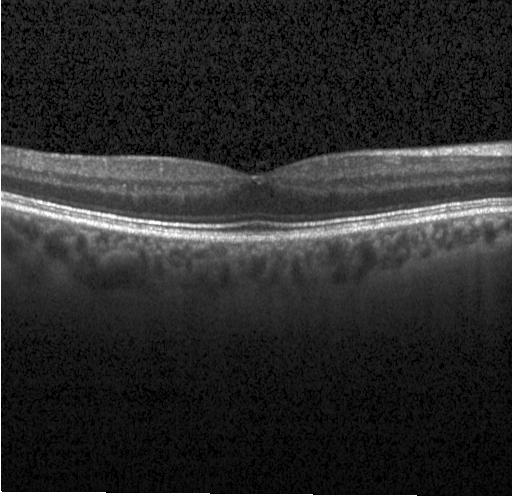 SD-OCT. Acquired on a Heidelberg Spectralis. Optical coherence tomography B-scan
The scan shows no evidence of choroidal neovascularization, diabetic macular edema, or drusen.